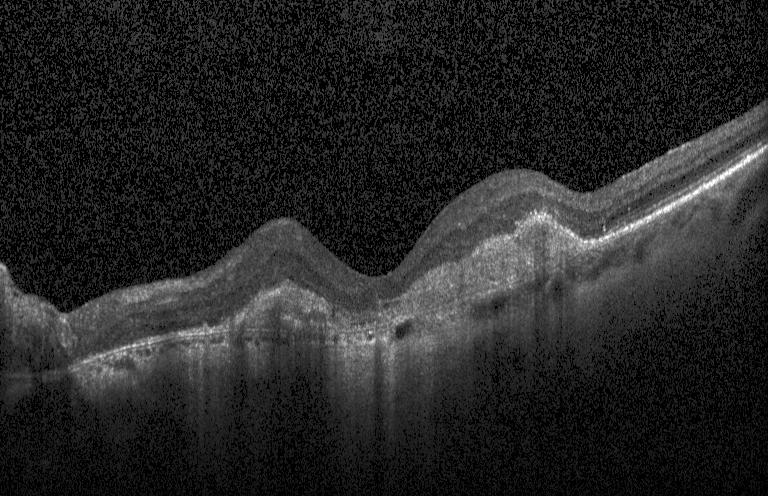

Heidelberg Spectralis, retinal OCT B-scan — The scan shows a choroidal neovascular membrane.